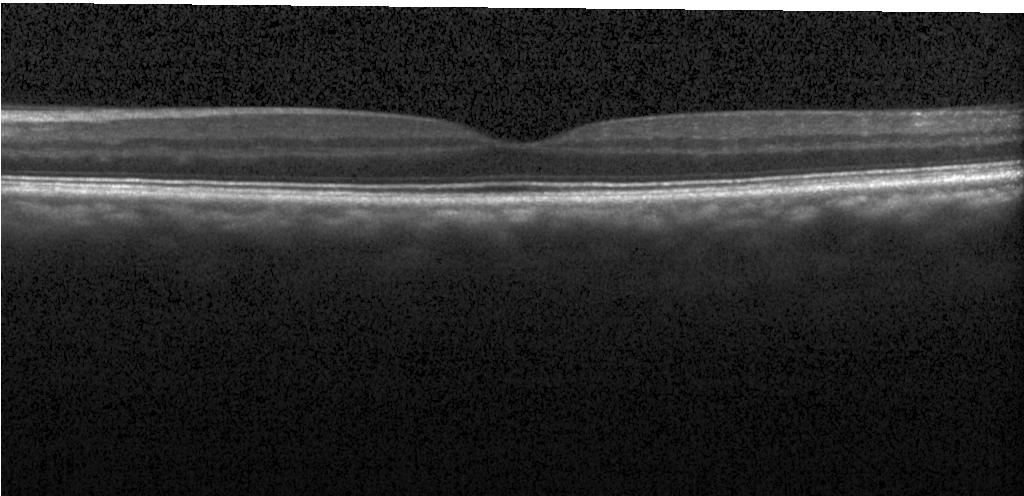

Optical coherence tomography B-scan, Heidelberg Spectralis OCT system.
No evidence of choroidal neovascularization, diabetic macular edema, or drusen.